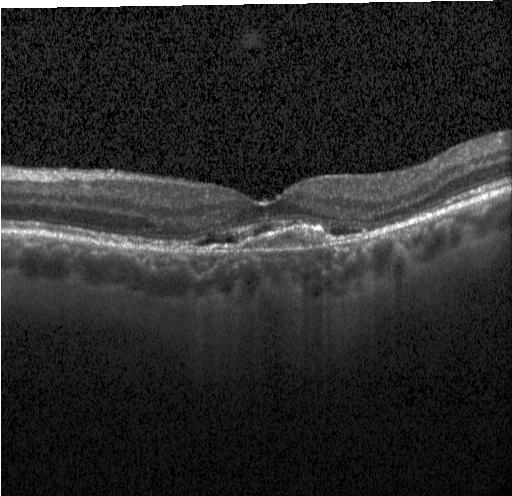 Retinal OCT cross-section showing a choroidal neovascular membrane.